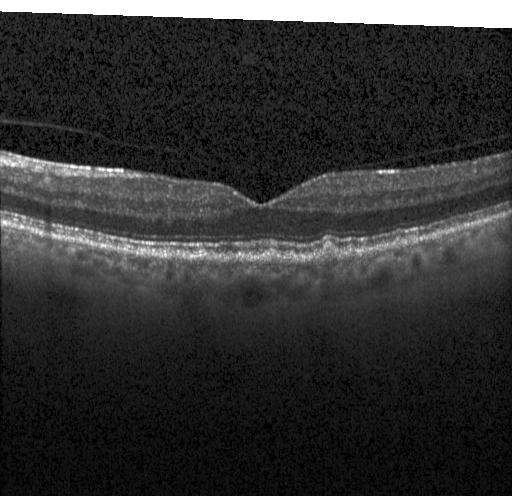
Macular OCT: sub-RPE drusenoid deposits.